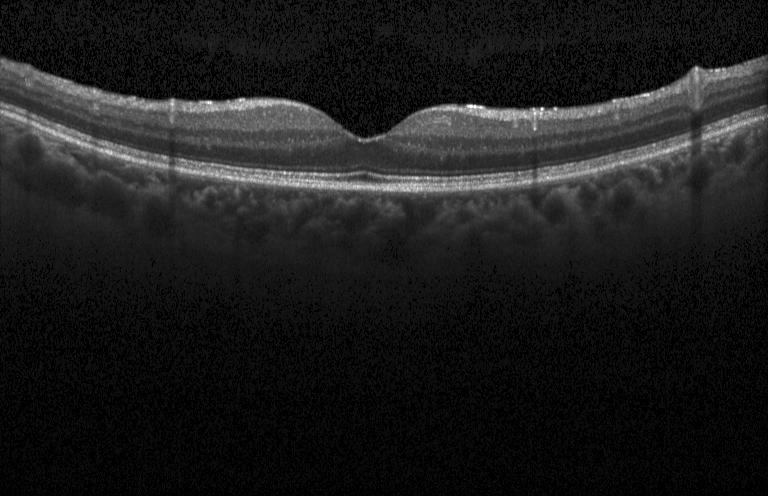 Impression: no choroidal neovascularization, diabetic macular edema, or drusen.